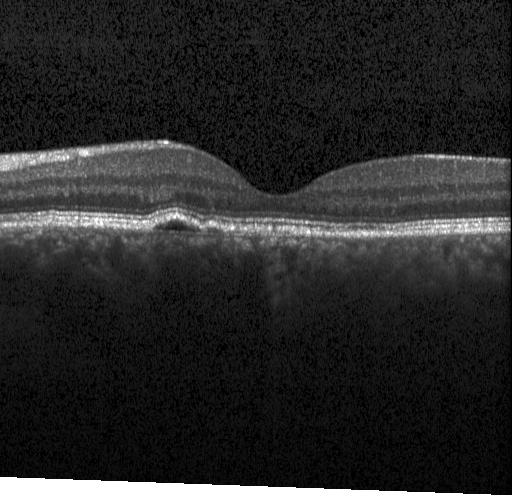 Macular OCT demonstrating choroidal neovascularization (CNV).